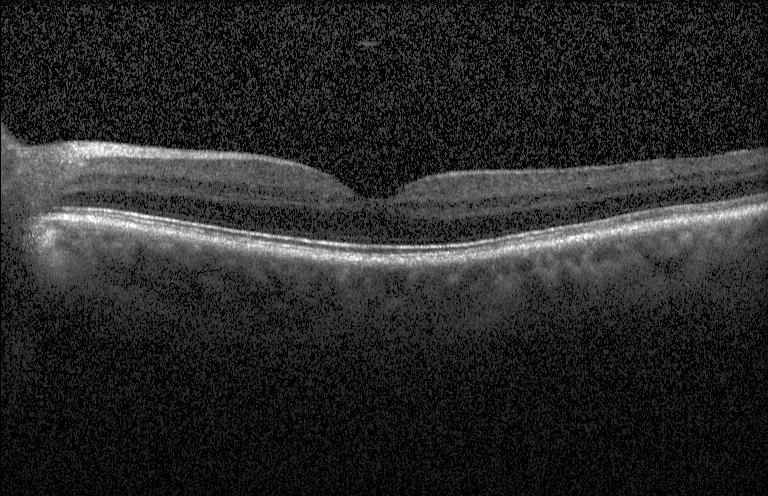 Finding: no choroidal neovascularization, no diabetic macular edema, and no drusen.